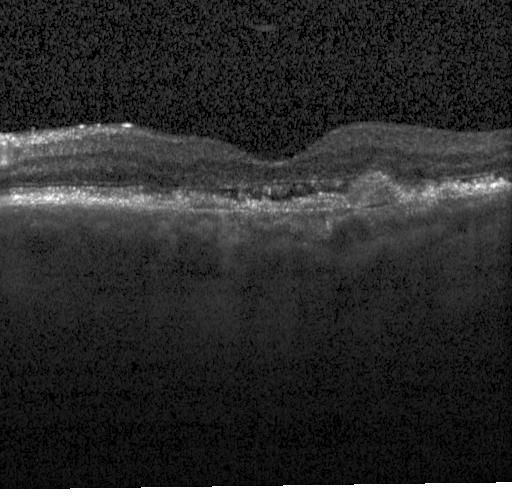

Optical coherence tomography scan. Heidelberg Spectralis. Diagnosis: CNV.